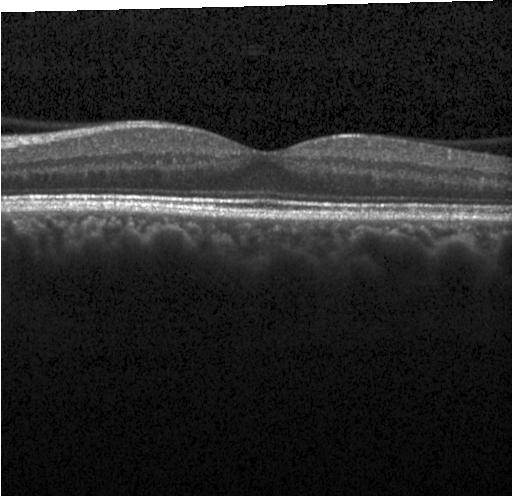

Finding: no choroidal neovascularization, diabetic macular edema, or drusen.